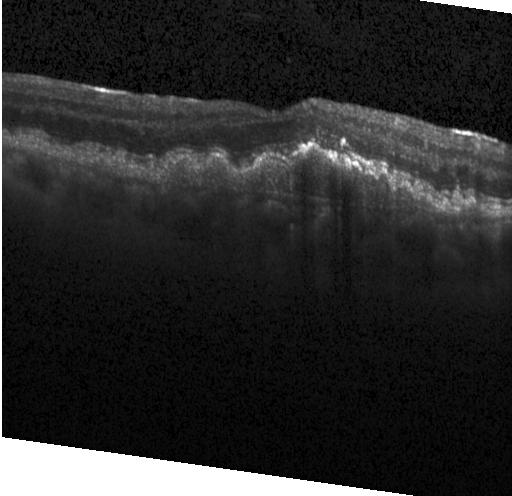 Assessment: a choroidal neovascular membrane.